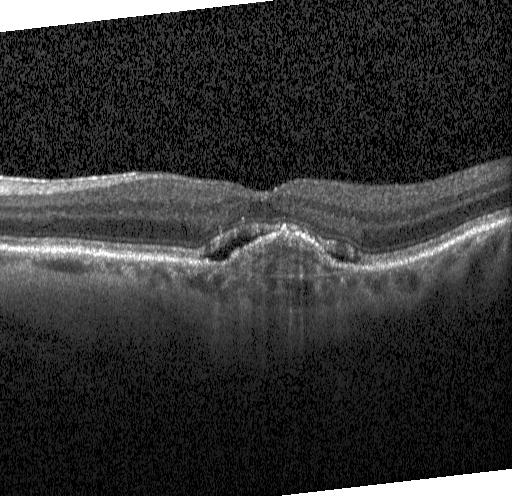

Spectral-domain OCT, OCT line scan. Finding: choroidal neovascularization (CNV).